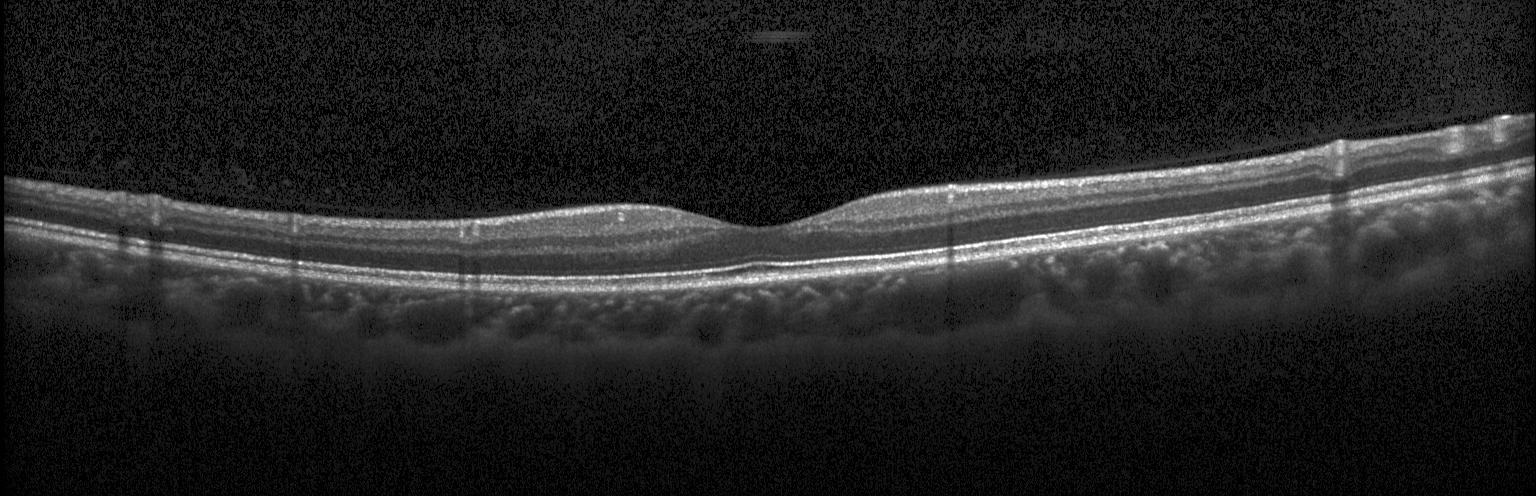 Spectral-domain optical coherence tomography. Through the macula. OCT line scan. Acquired on a Heidelberg Spectralis
Macular OCT: neither choroidal neovascularization, diabetic macular edema, nor drusen.